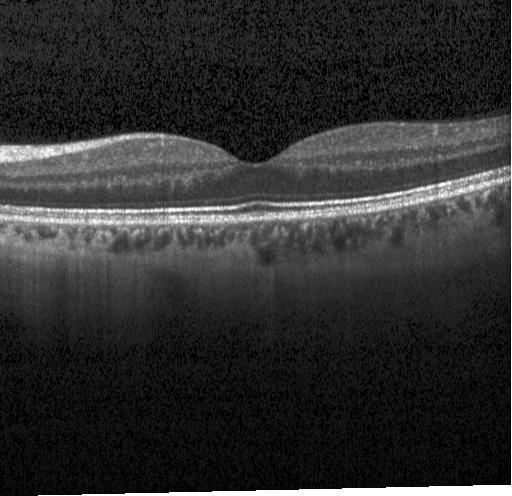

Spectral-domain OCT, instrument: Heidelberg Spectralis, optical coherence tomography scan.
This B-scan demonstrates neither choroidal neovascularization, diabetic macular edema, nor drusen.